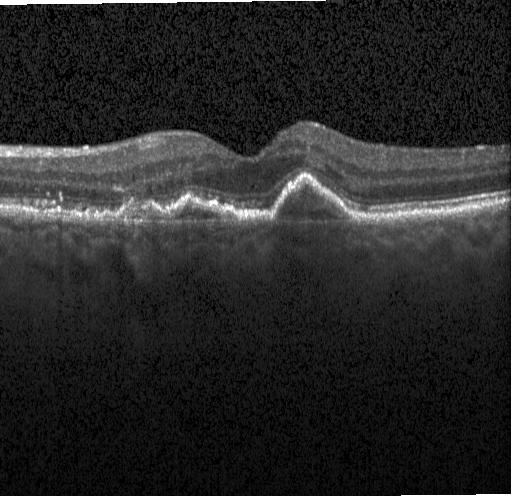
Centered on the fovea. OCT line scan — The scan shows choroidal neovascularization.